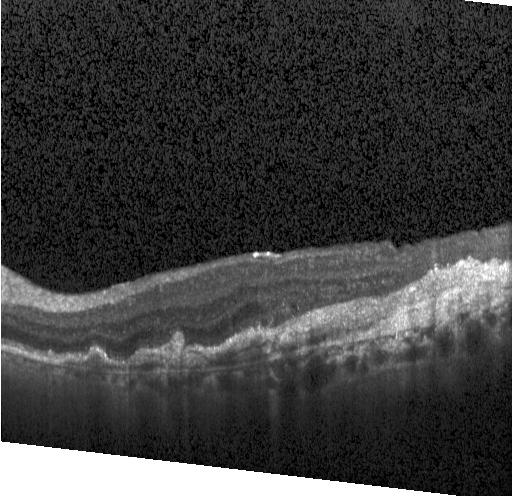 The scan shows a choroidal neovascular membrane.